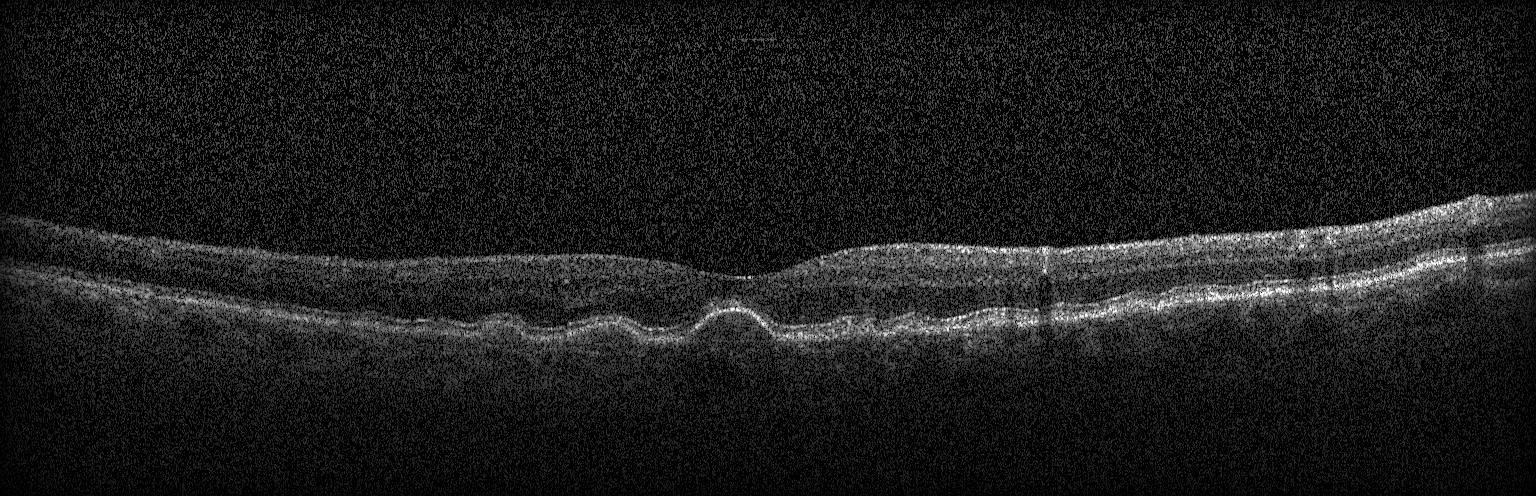 OCT line scan. Multiple drusen.